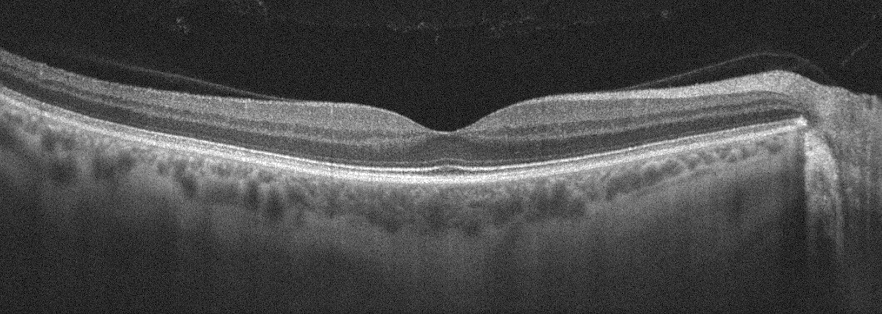 Macular scan; Optovue Avanti RTVue XR; retinal OCT B-scan — OCT finding: absence of AMD, DME, ERM, RAO, RVO, and vitreomacular interface disease.